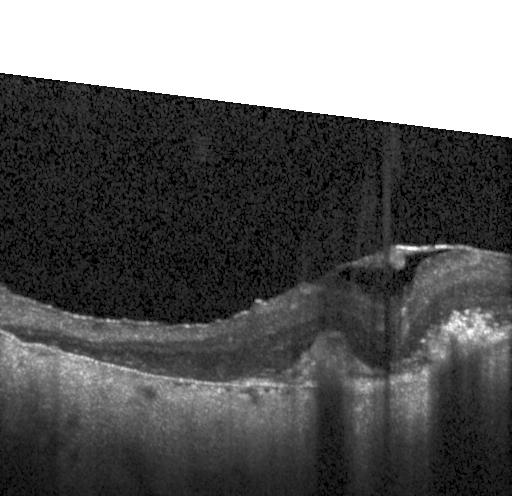 Retinal OCT B-scan · spectral-domain optical coherence tomography · fovea-centered.
Finding: choroidal neovascularization (CNV).